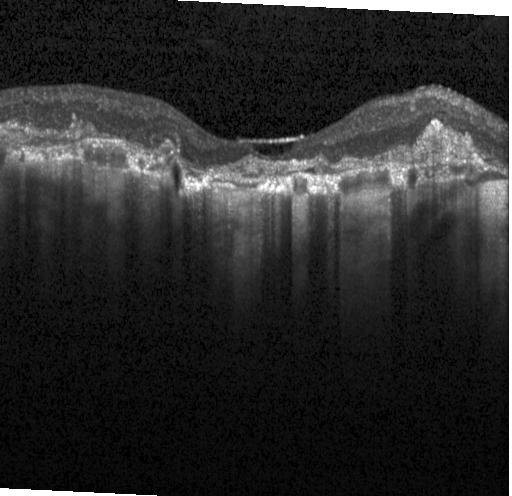 OCT B-scan. Acquired on a Heidelberg Spectralis. Impression: a choroidal neovascular membrane.